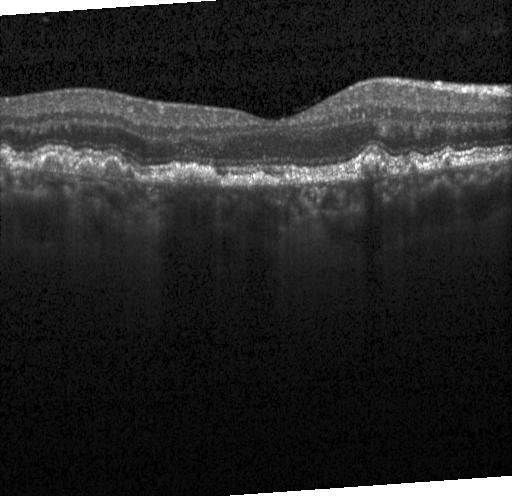

OCT line scan. Acquired on a Heidelberg Spectralis. Spectral-domain optical coherence tomography. Horizontal scan through the fovea
Impression: sub-RPE drusenoid deposits.